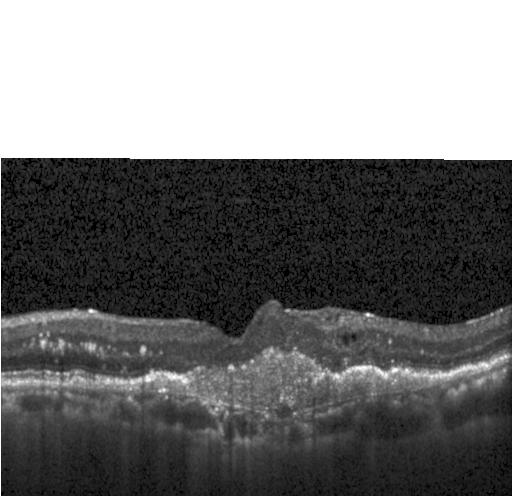

Horizontal scan through the fovea, acquired on a Heidelberg Spectralis, optical coherence tomography B-scan
Finding: a choroidal neovascular membrane.